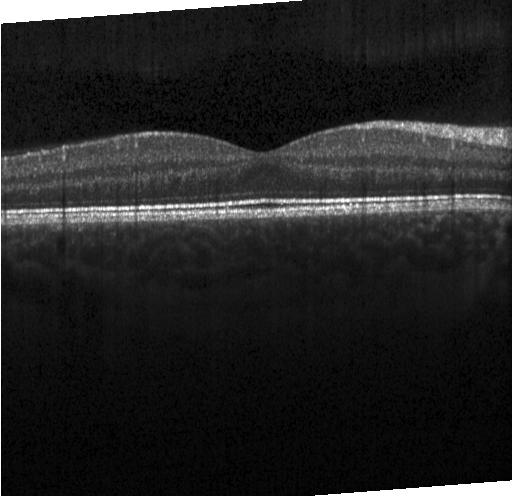

Finding: no evidence of choroidal neovascularization, diabetic macular edema, or drusen.